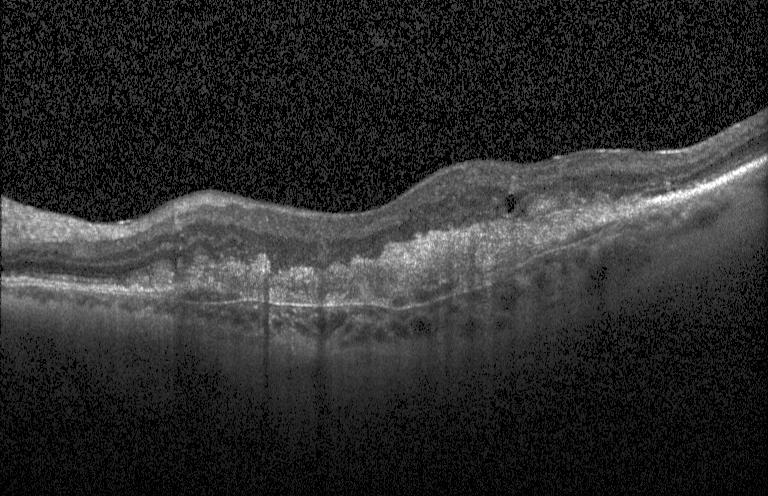
Diagnosis: a choroidal neovascular membrane.